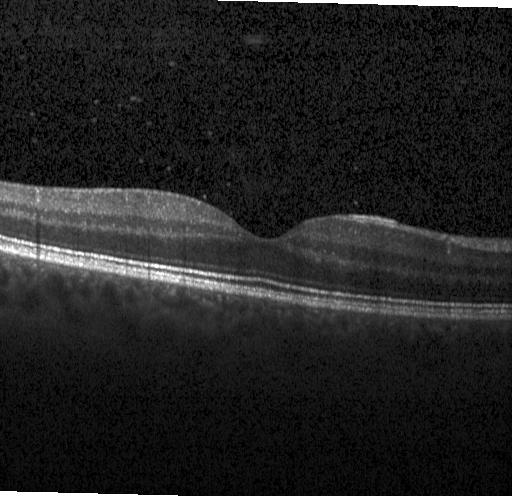
OCT finding: no CNV, DME, or drusen.